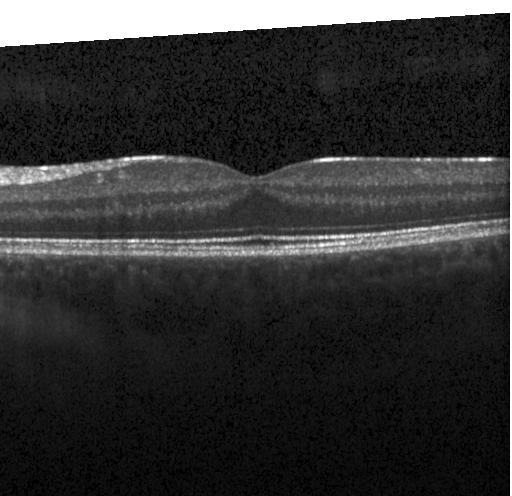 Spectral-domain OCT. Retinal OCT B-scan — This B-scan demonstrates no choroidal neovascularization, diabetic macular edema, or drusen.